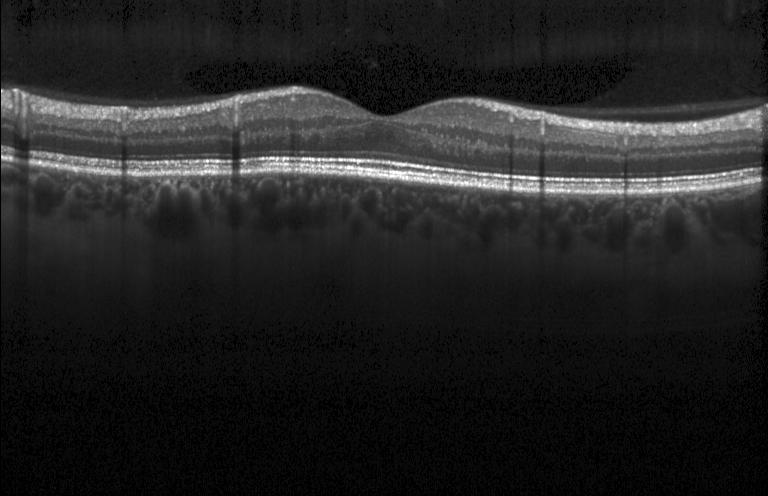 The scan shows no evidence of CNV, DME, or drusen.